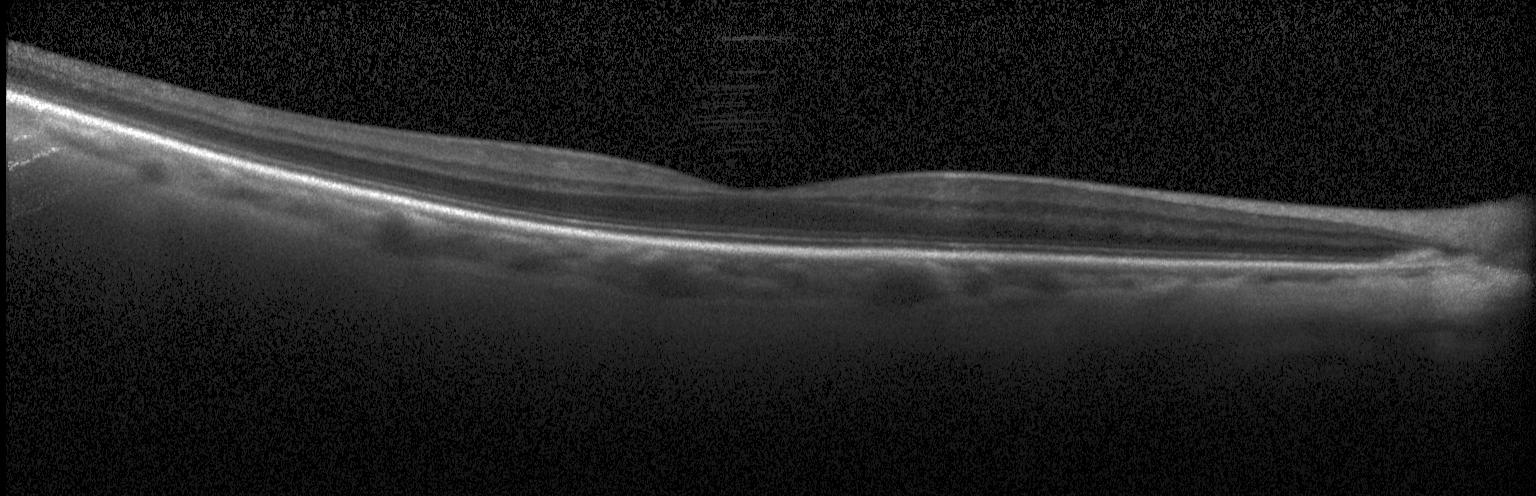
OCT B-scan showing no evidence of choroidal neovascularization, diabetic macular edema, or drusen.